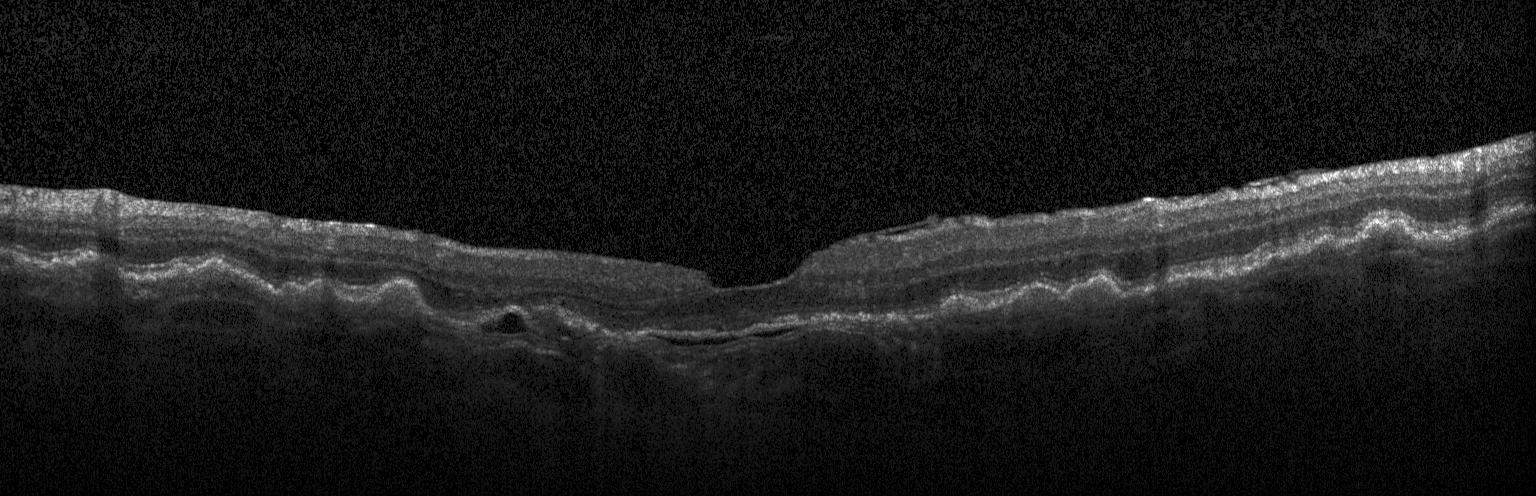 Diagnosis: choroidal neovascularization (CNV).